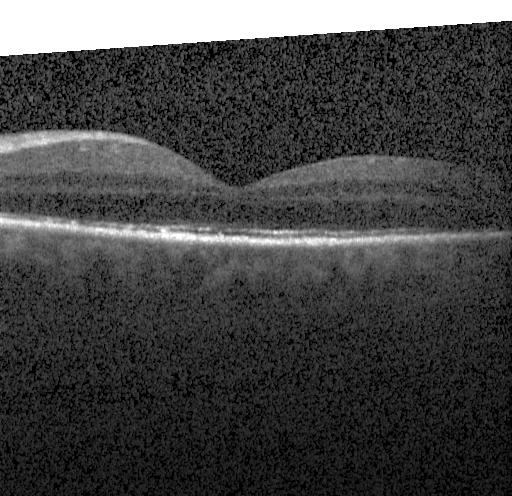 Macular OCT demonstrating neither CNV, DME, nor drusen.